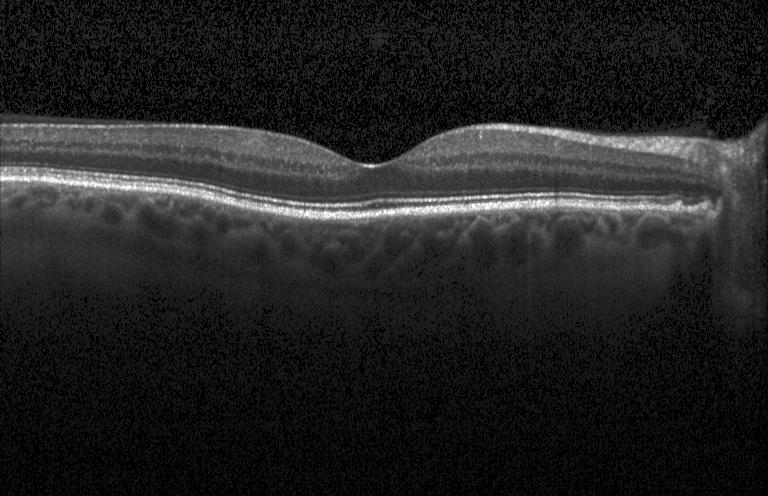
Optical coherence tomography scan; Heidelberg Spectralis; fovea-centered; spectral-domain optical coherence tomography.
Diagnosis: neither choroidal neovascularization, diabetic macular edema, nor drusen.